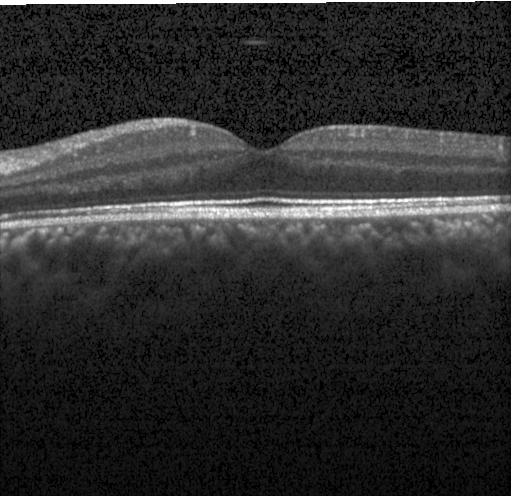

Optical coherence tomography scan
Diagnosis: no choroidal neovascularization, no diabetic macular edema, and no drusen.